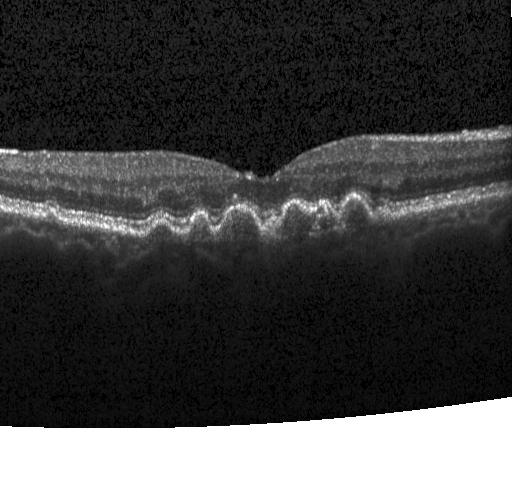
Assessment: sub-RPE drusenoid deposits.